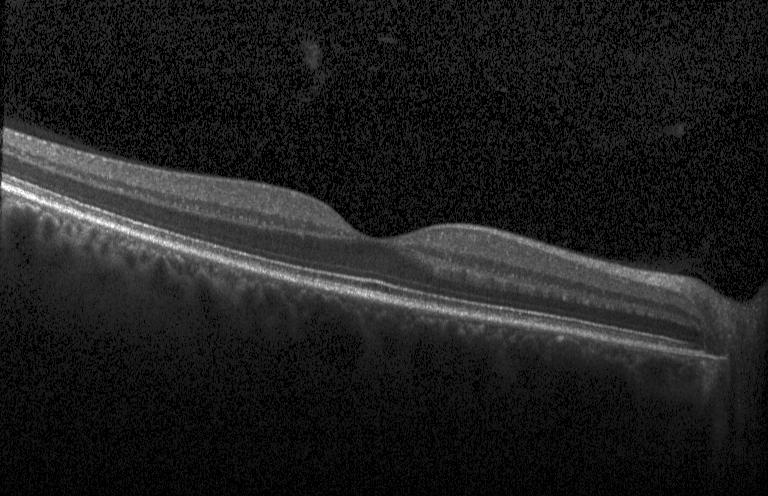 Retinal OCT cross-section.
OCT finding: no choroidal neovascularization, no diabetic macular edema, and no drusen.